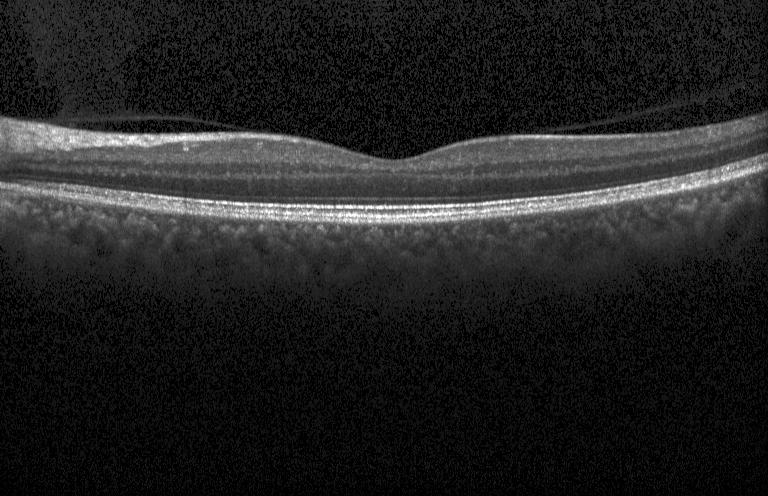

Retinal OCT cross-section showing no choroidal neovascularization, no diabetic macular edema, and no drusen.